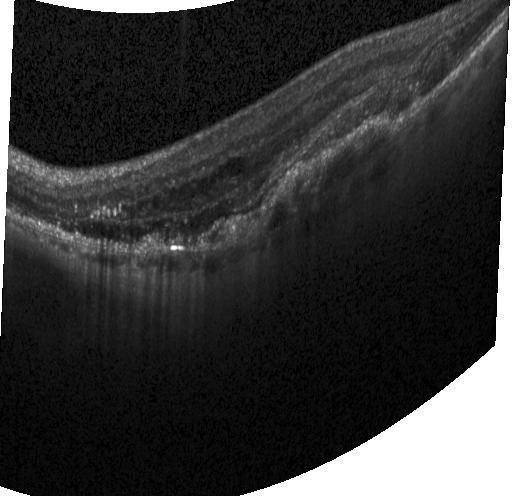 OCT B-scan showing a choroidal neovascular membrane.